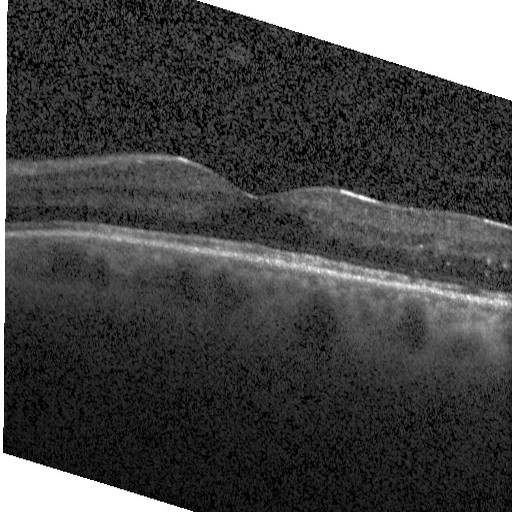 OCT line scan; spectral-domain OCT; acquired on a Heidelberg Spectralis — Macular OCT: DME.